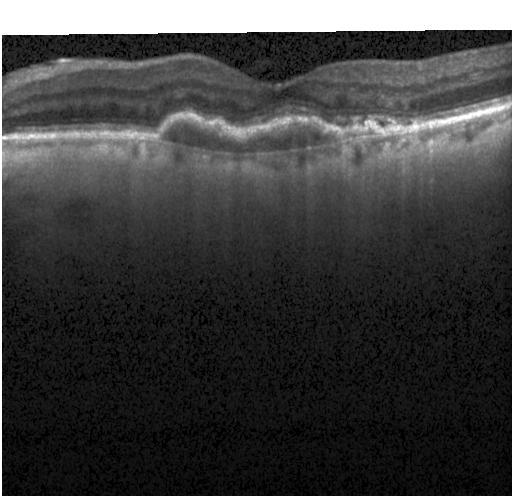
Retinal OCT cross-section showing a choroidal neovascular membrane.